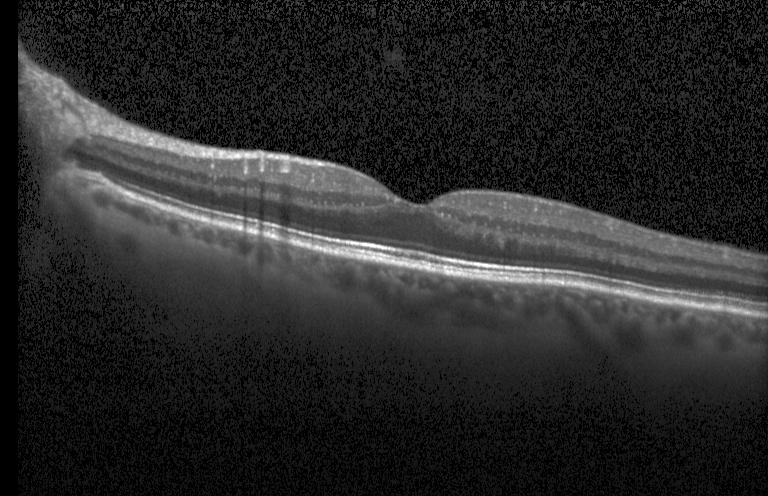
Centered on the fovea; retinal OCT B-scan; spectral-domain optical coherence tomography; instrument: Heidelberg Spectralis.
Macular OCT: neither choroidal neovascularization, diabetic macular edema, nor drusen.